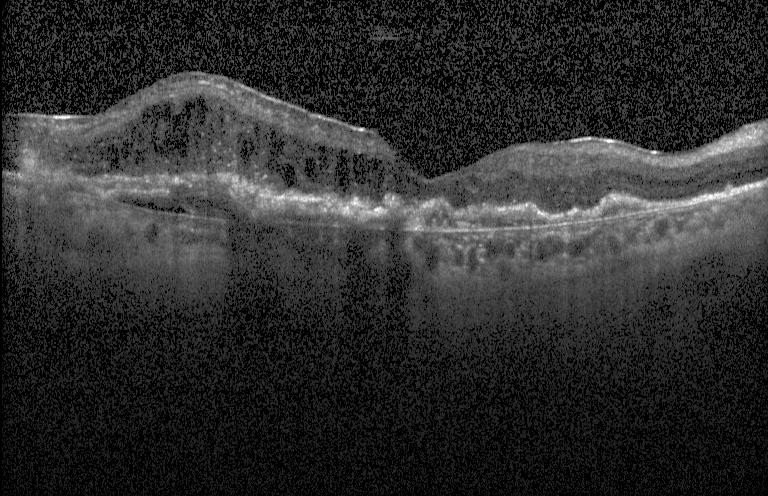 Spectral-domain optical coherence tomography. Through the macula. OCT line scan — Assessment: a choroidal neovascular membrane.